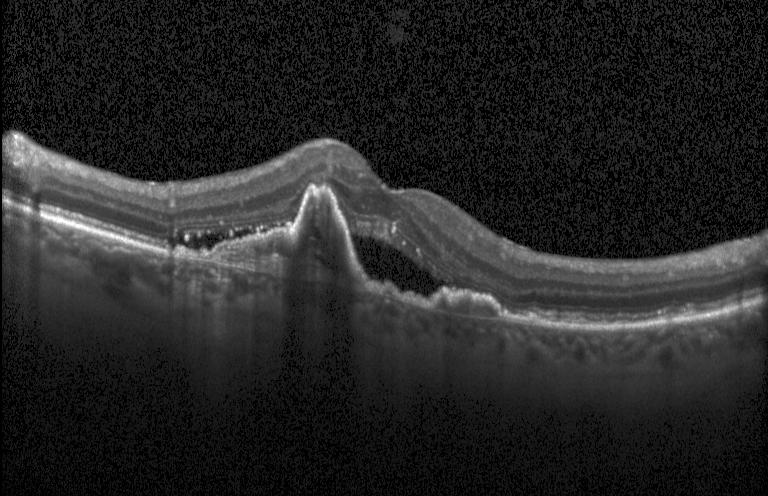

Retinal OCT cross-section showing CNV.